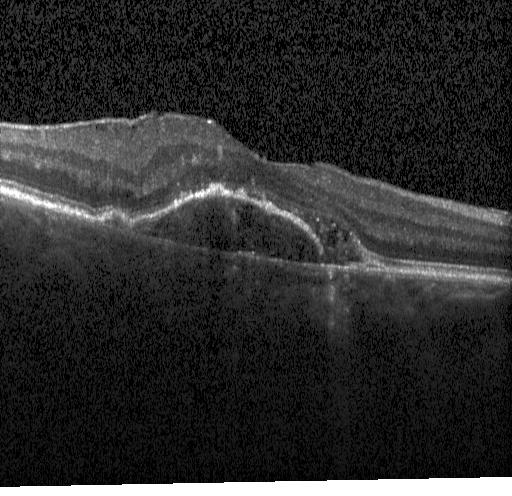

Retinal OCT cross-section showing choroidal neovascularization.